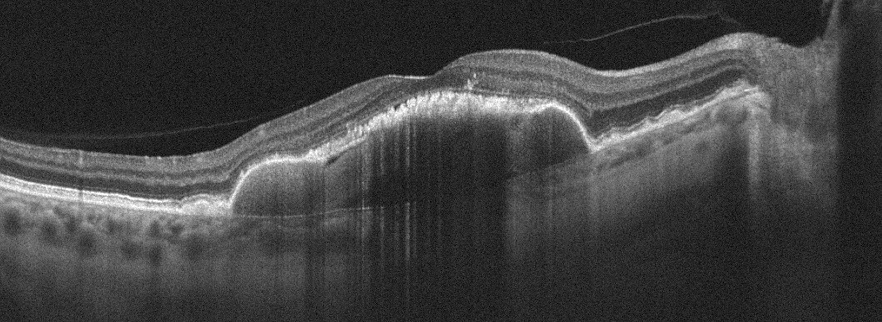

Fovea-centered; optical coherence tomography B-scan
Impression: AMD.